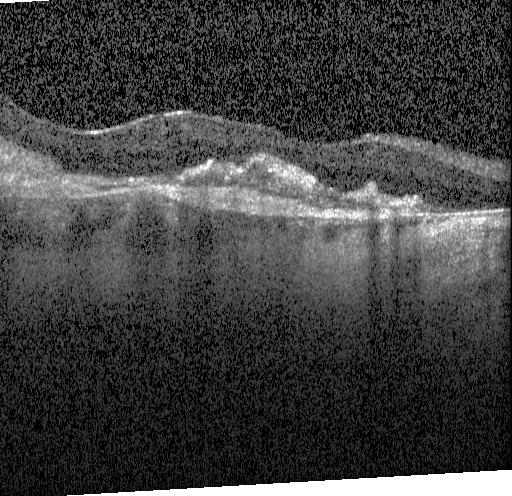

Optical coherence tomography B-scan, spectral-domain optical coherence tomography, centered on the fovea, acquired on a Heidelberg Spectralis.
Dx: a choroidal neovascular membrane.